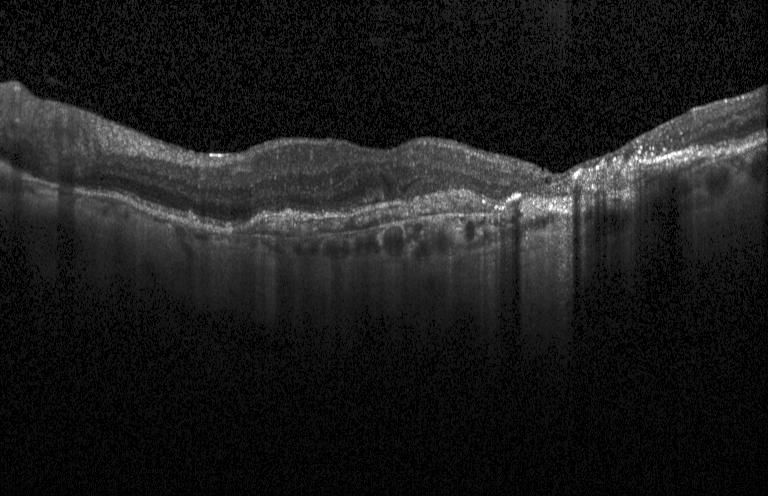

OCT line scan · horizontal scan through the fovea · Heidelberg Spectralis OCT system.
Finding: choroidal neovascularization (CNV).